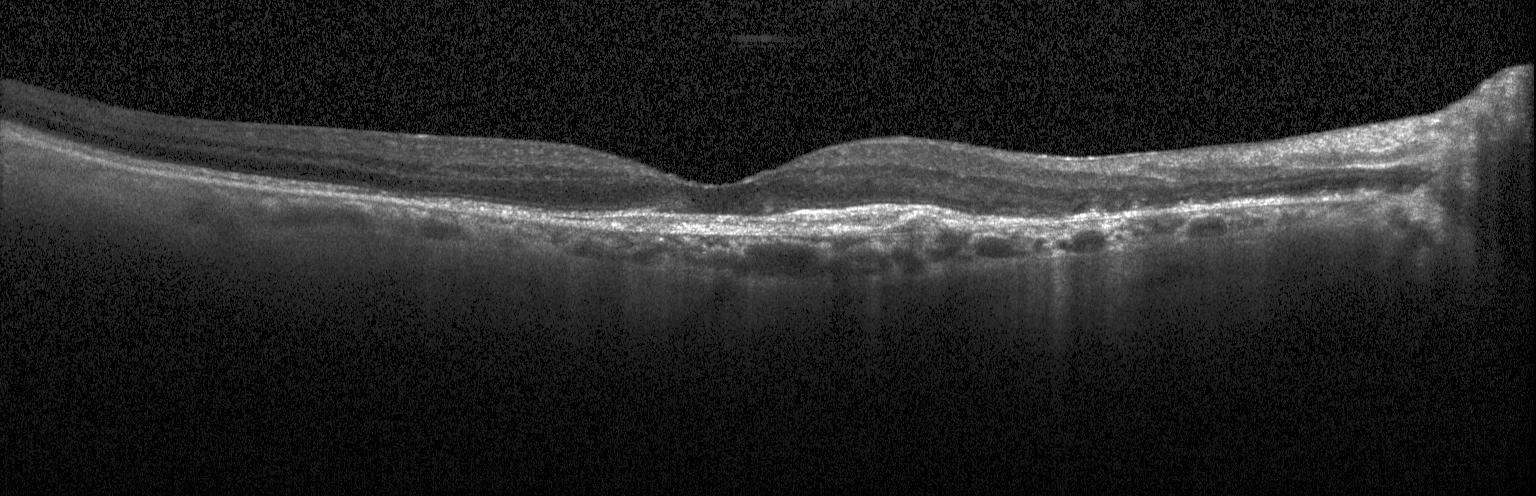

Macular OCT: choroidal neovascularization (CNV).